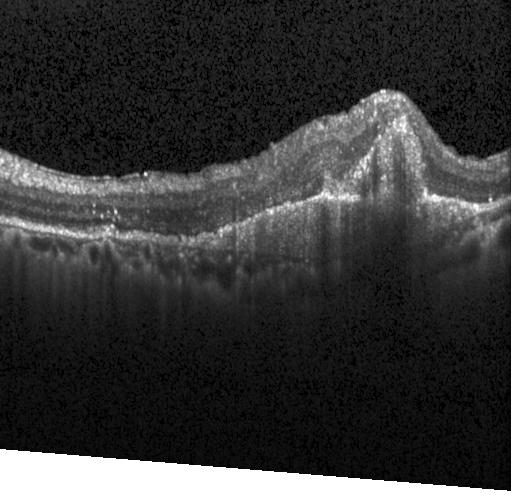
Heidelberg Spectralis. Spectral-domain optical coherence tomography. Macular scan. Optical coherence tomography scan
Impression: choroidal neovascularization.